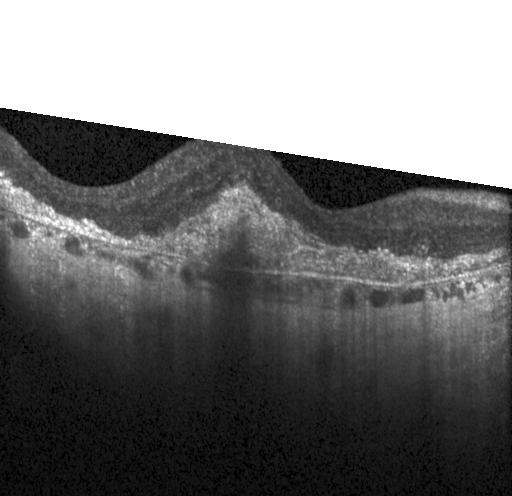 Diagnosis: a choroidal neovascular membrane.